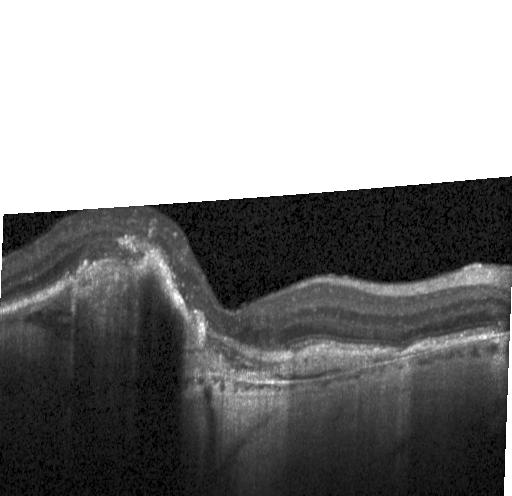

OCT B-scan. Impression: a choroidal neovascular membrane.